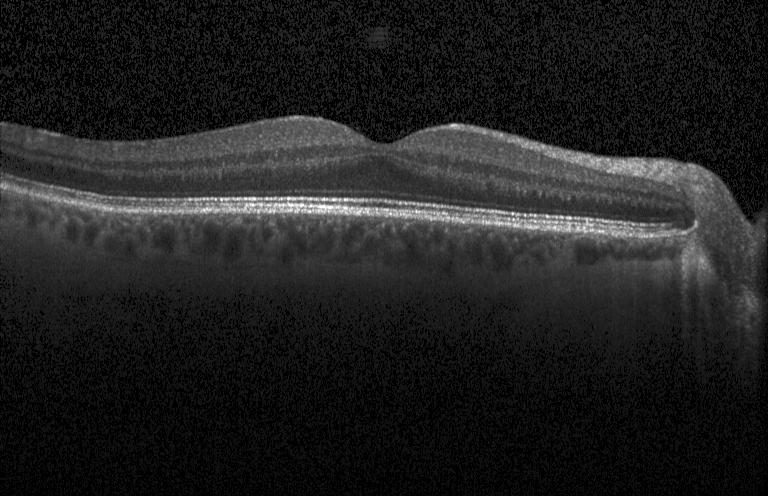
Spectral-domain optical coherence tomography · macular scan · optical coherence tomography B-scan
The scan shows neither CNV, DME, nor drusen.